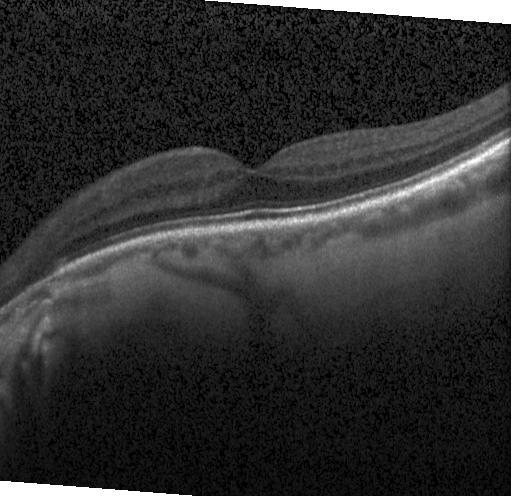
Heidelberg Spectralis; optical coherence tomography scan; spectral-domain OCT; horizontal scan through the fovea
Impression: no evidence of choroidal neovascularization, diabetic macular edema, or drusen.